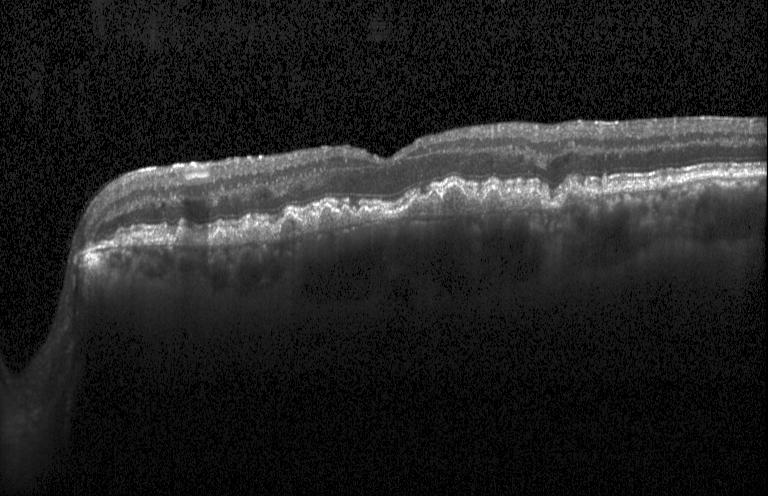 Centered on the fovea · Heidelberg Spectralis OCT system · retinal OCT B-scan. Finding: CNV.